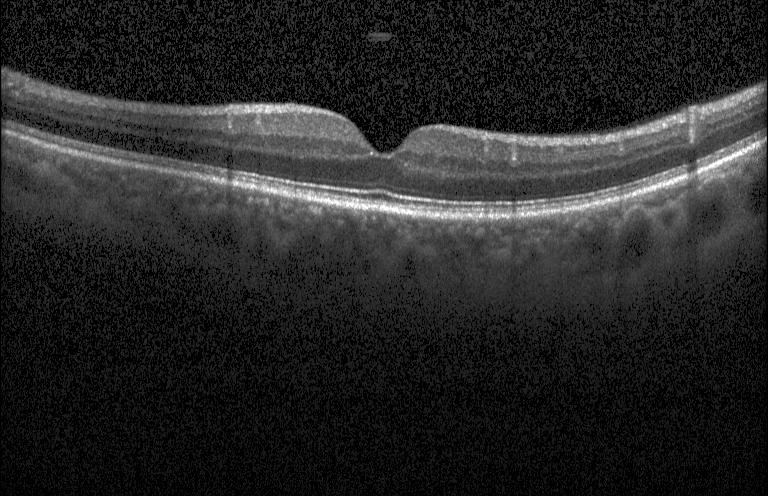
The scan shows no CNV, DME, or drusen.